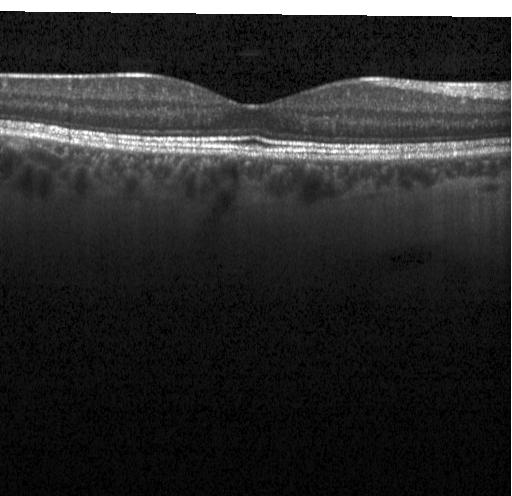 Optical coherence tomography scan. SD-OCT. Dx: no choroidal neovascularization, diabetic macular edema, or drusen.